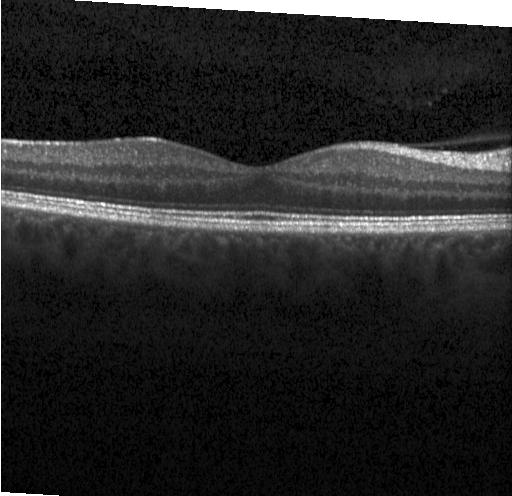
Horizontal scan through the fovea. Retinal OCT cross-section — Impression: neither choroidal neovascularization, diabetic macular edema, nor drusen.